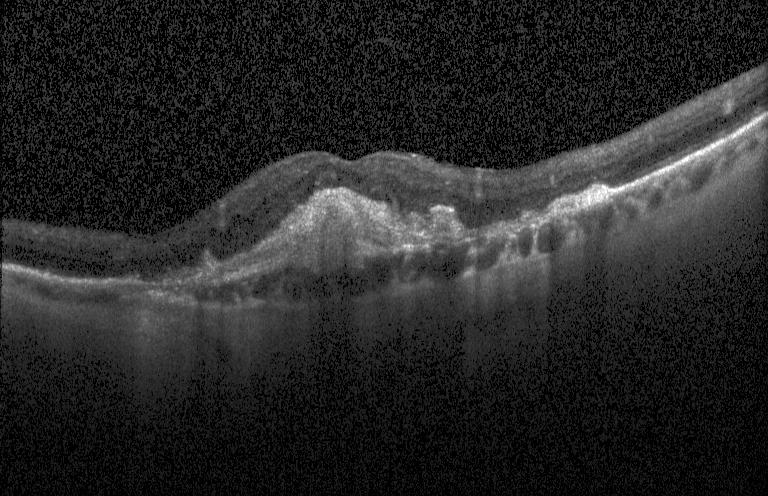 Instrument: Heidelberg Spectralis. OCT B-scan. Fovea-centered. Spectral-domain OCT.
Finding: choroidal neovascularization (CNV).